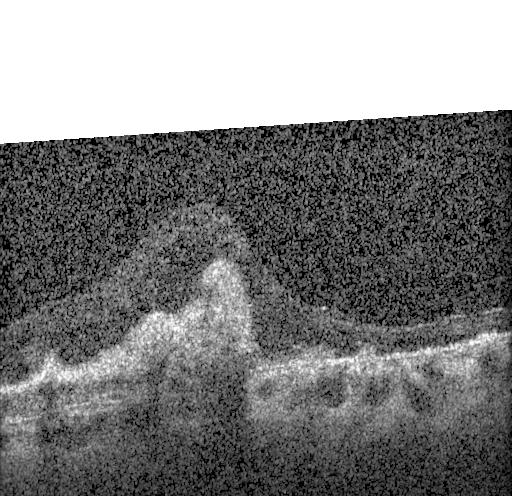
OCT finding: a choroidal neovascular membrane.